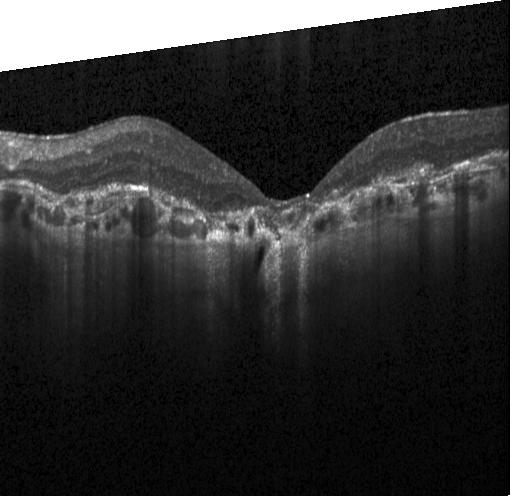 Instrument: Heidelberg Spectralis. OCT line scan. Fovea-centered.
Diagnosis: a choroidal neovascular membrane.